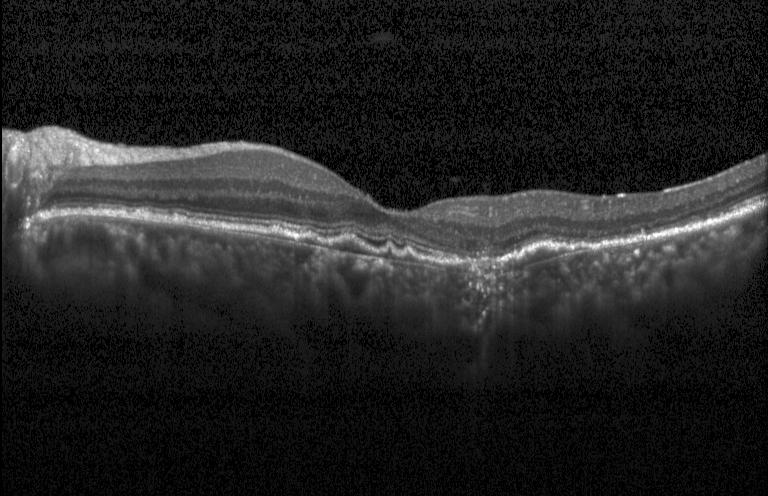

The scan shows a choroidal neovascular membrane.